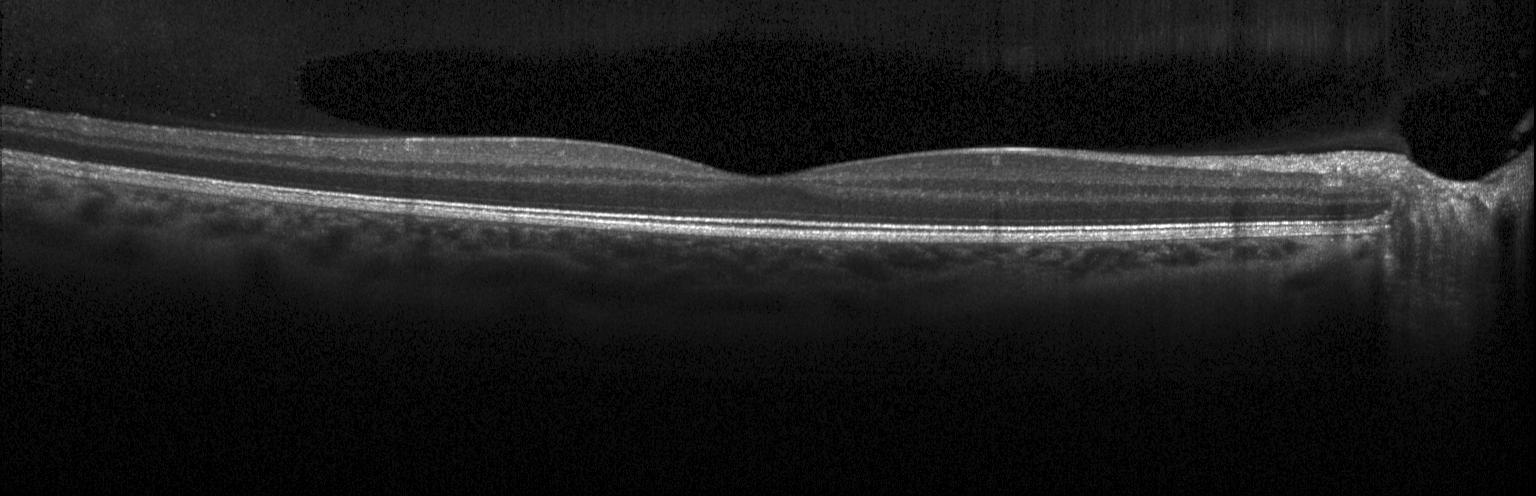

SD-OCT · optical coherence tomography scan. Diagnosis: no CNV, no DME, and no drusen.